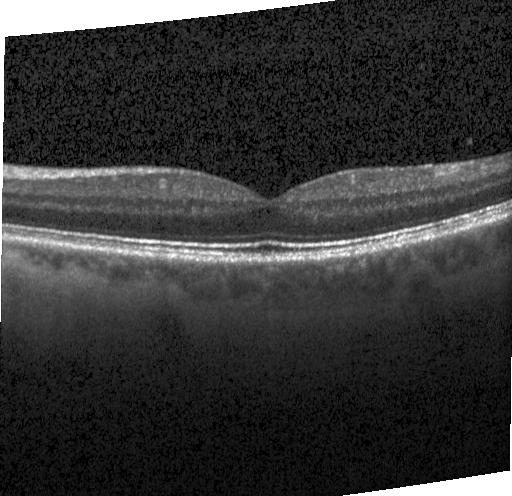

Spectral-domain optical coherence tomography. Optical coherence tomography scan. Centered on the fovea — Diagnosis: neither CNV, DME, nor drusen.